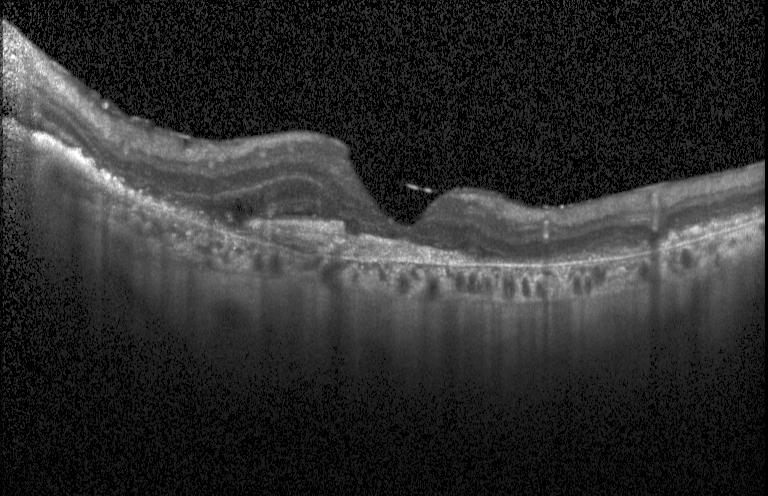
Dx: CNV.